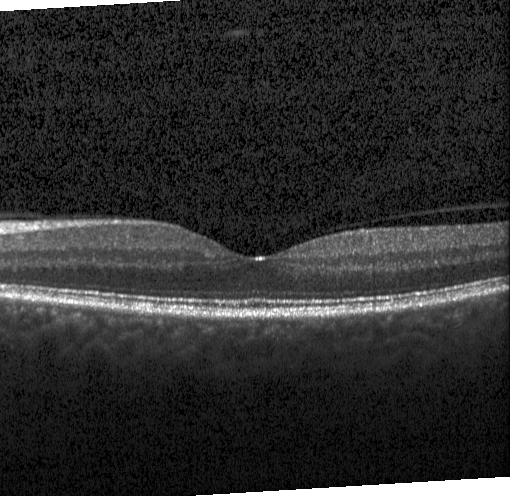

Spectral-domain OCT · Heidelberg Spectralis OCT system · macular scan · OCT B-scan.
Finding: no evidence of choroidal neovascularization, diabetic macular edema, or drusen.